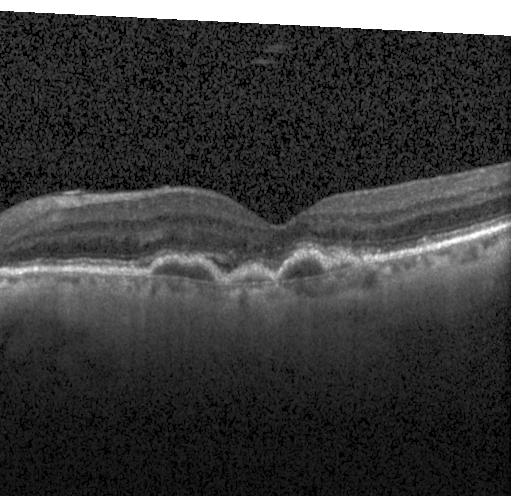 OCT line scan; centered on the fovea — OCT finding: a choroidal neovascular membrane.